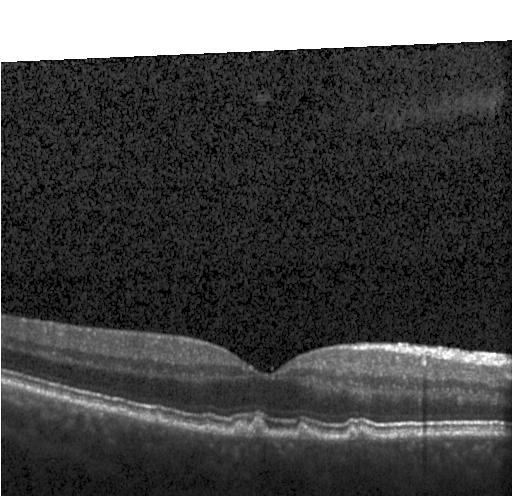 OCT B-scan
Finding: drusen.